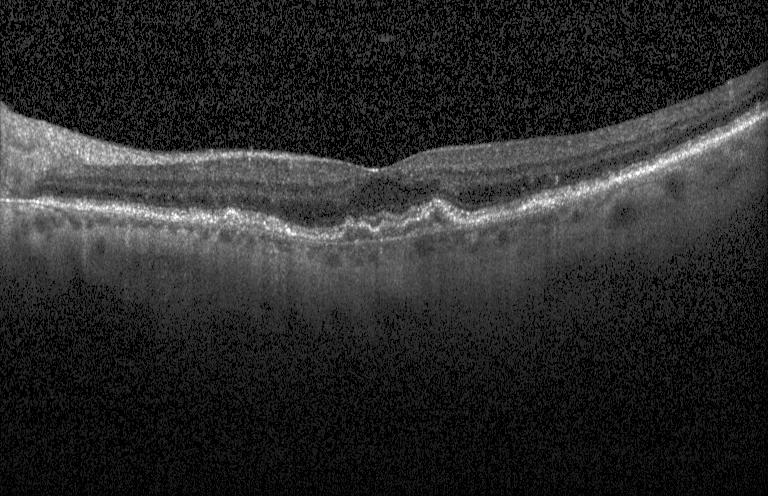

Optical coherence tomography B-scan, centered on the fovea.
Assessment: a choroidal neovascular membrane.